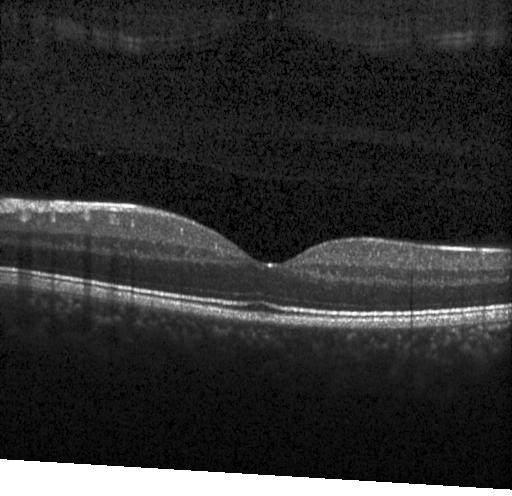 Retinal OCT cross-section showing no evidence of choroidal neovascularization, diabetic macular edema, or drusen.